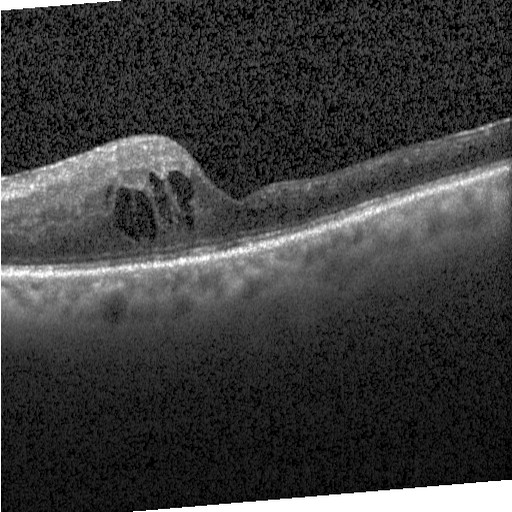

OCT B-scan, instrument: Heidelberg Spectralis.
Macular OCT: diabetic macular edema (DME).